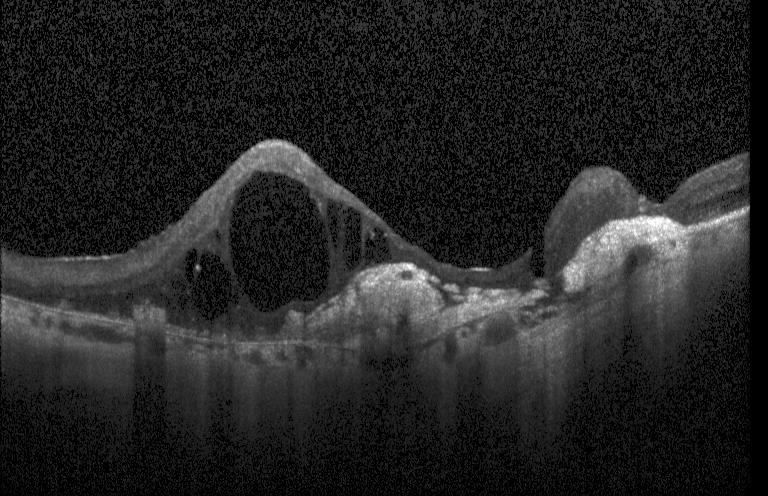

SD-OCT · Heidelberg Spectralis OCT system · OCT line scan
Dx: a choroidal neovascular membrane.